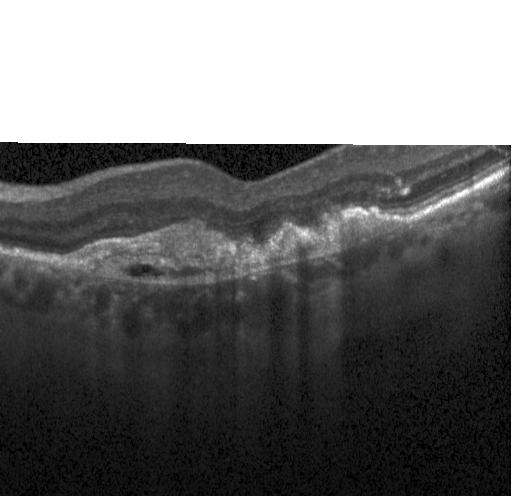

Retinal OCT B-scan, centered on the fovea, instrument: Heidelberg Spectralis. Assessment: a choroidal neovascular membrane.